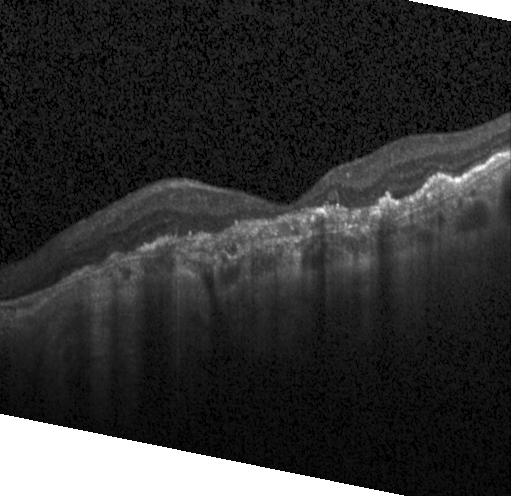 The scan shows a choroidal neovascular membrane.